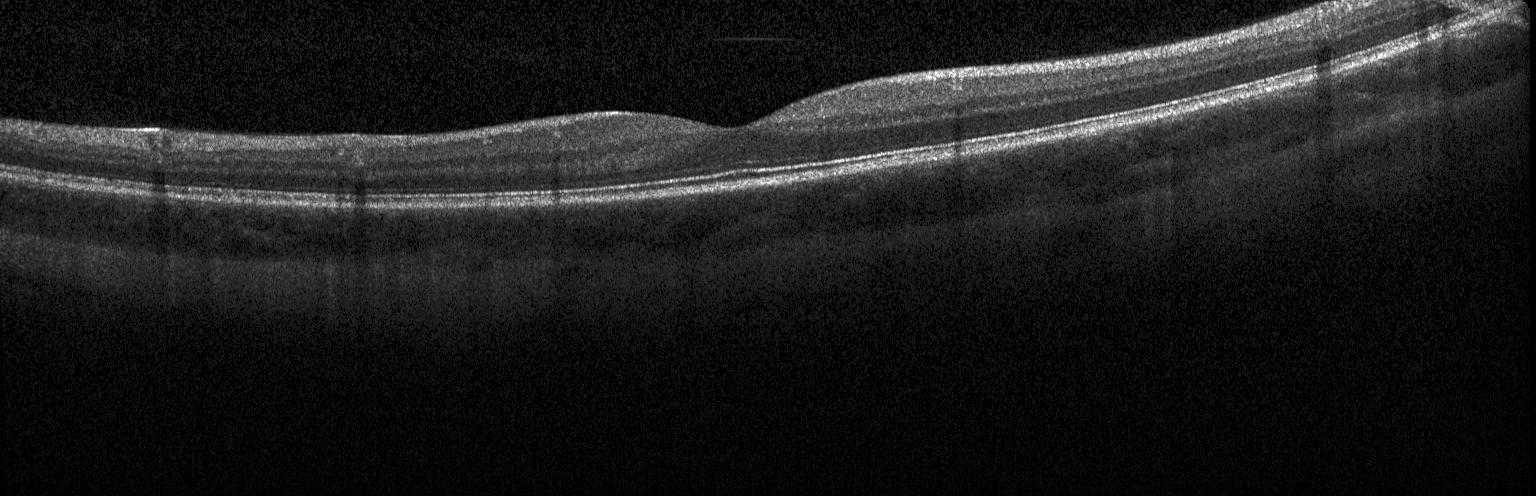

Optical coherence tomography scan — Macular OCT: neither CNV, DME, nor drusen.